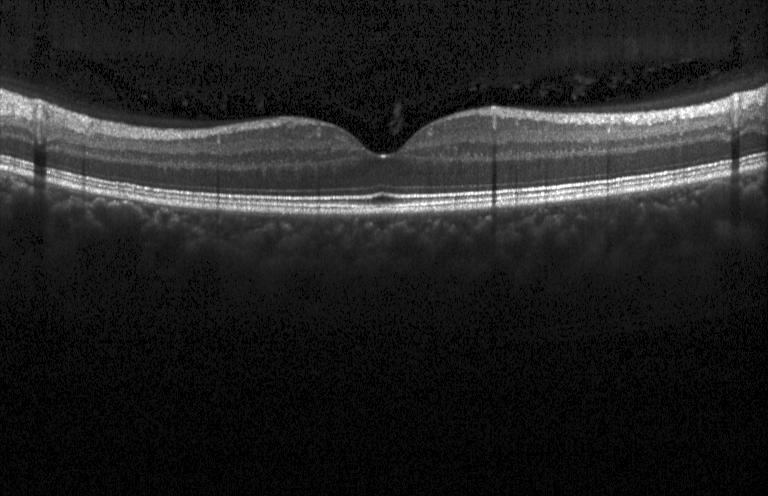

Macular scan, optical coherence tomography scan — Impression: no CNV, DME, or drusen.